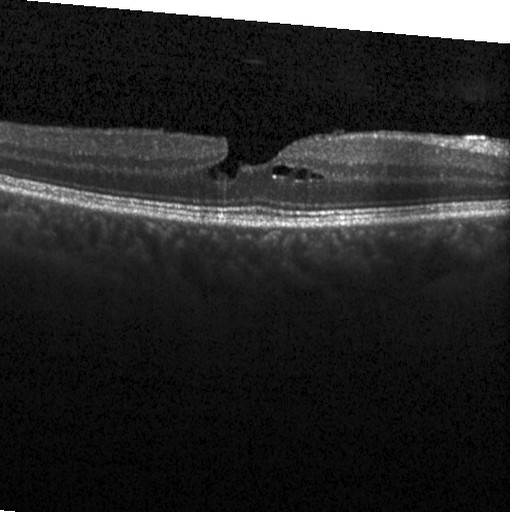 Centered on the fovea · retinal OCT cross-section · SD-OCT · acquired on a Heidelberg Spectralis
Impression: diabetic macular edema.